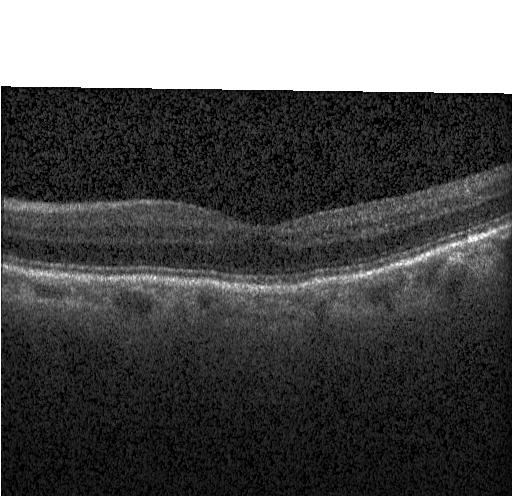 Spectral-domain optical coherence tomography. Instrument: Heidelberg Spectralis. OCT B-scan. Centered on the fovea
Impression: no choroidal neovascularization, diabetic macular edema, or drusen.